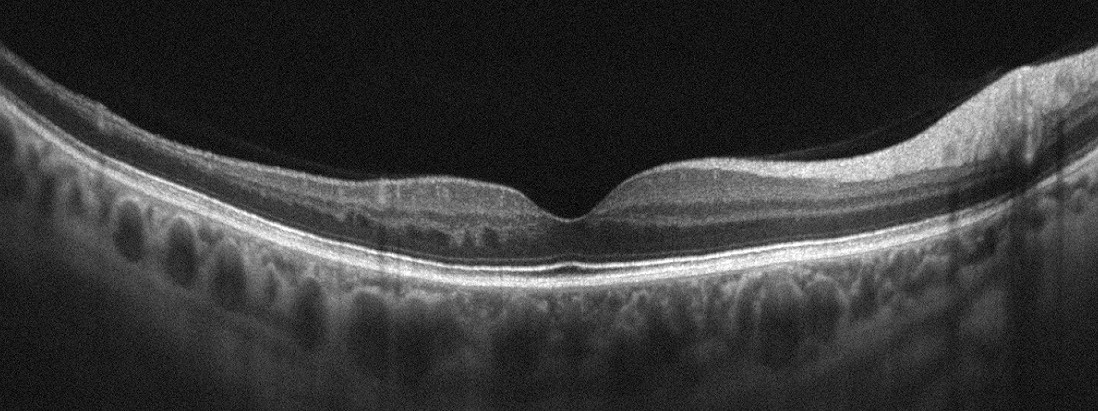
Retinal OCT cross-section. Through the macula — Impression: RVO.